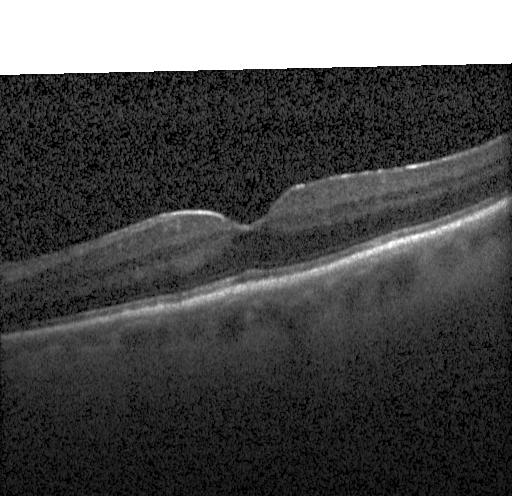
Impression: no choroidal neovascularization, diabetic macular edema, or drusen.